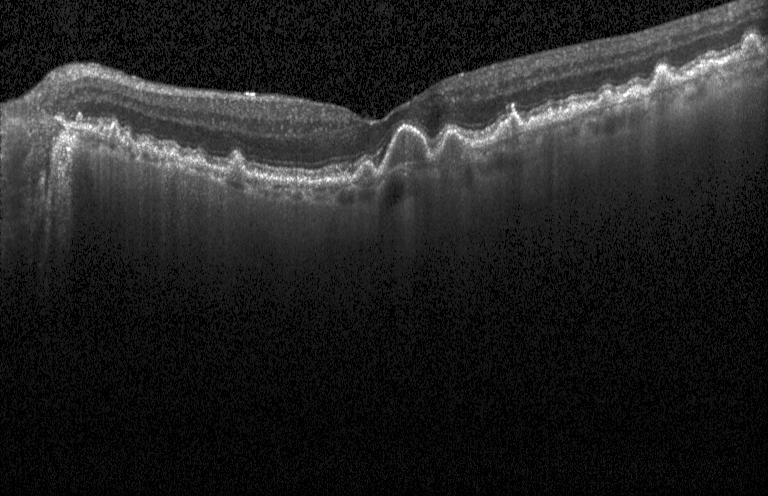

Macular OCT demonstrating multiple drusen.